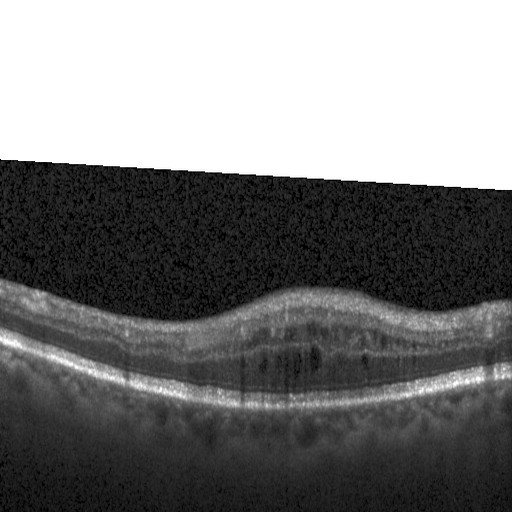
Diagnosis: diabetic macular edema (DME).